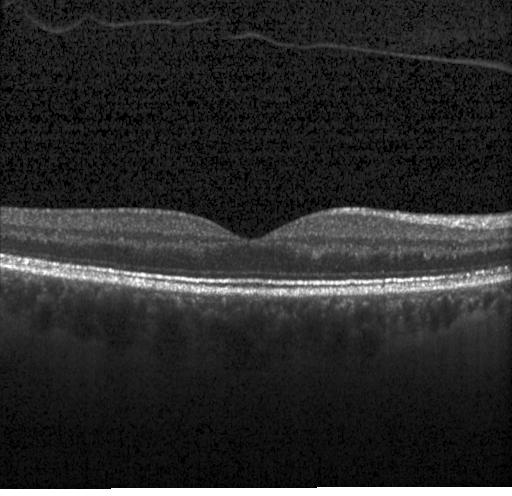

Diagnosis: no choroidal neovascularization, diabetic macular edema, or drusen.